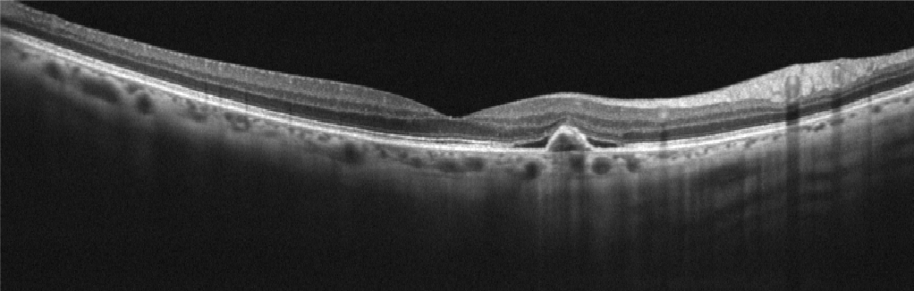

Assessment: age-related macular degeneration (AMD).